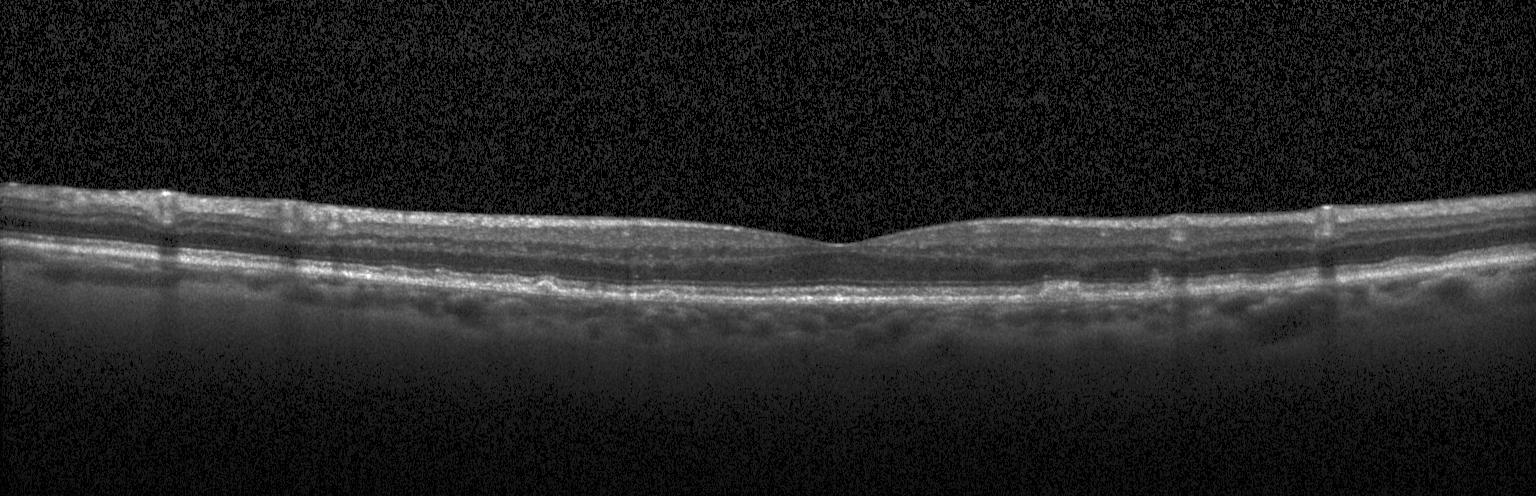 Assessment: sub-RPE drusenoid deposits.